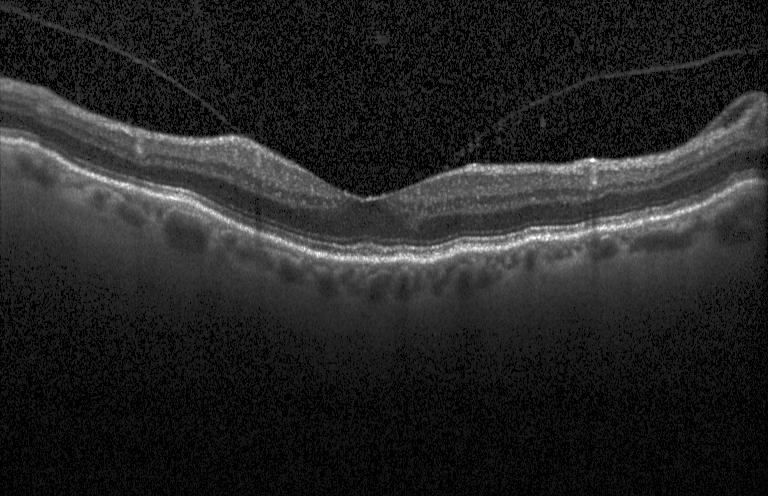 OCT finding: no choroidal neovascularization, no diabetic macular edema, and no drusen.